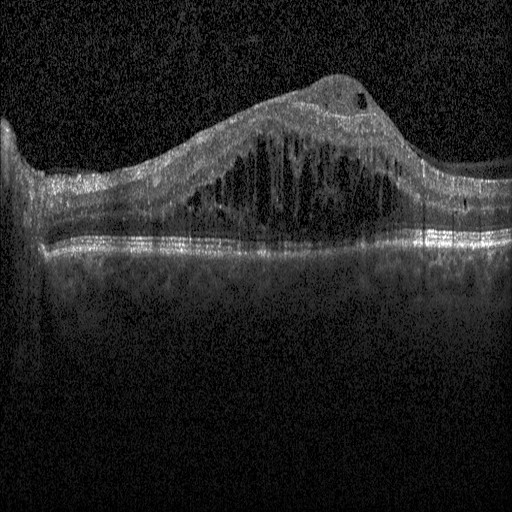 Optical coherence tomography B-scan, Heidelberg Spectralis OCT system — Diagnosis: DME.